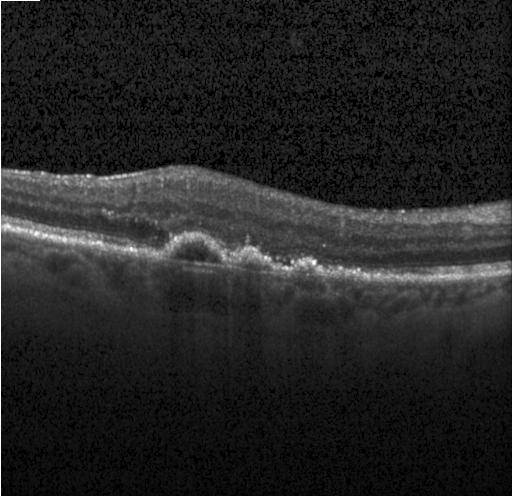 Optical coherence tomography scan. Spectral-domain optical coherence tomography. Fovea-centered
Diagnosis: a choroidal neovascular membrane.